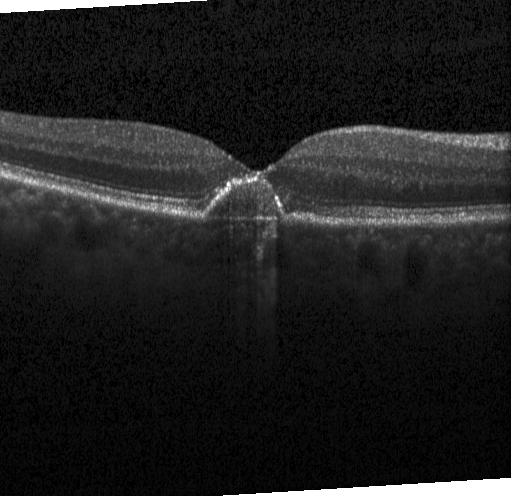
CNV.